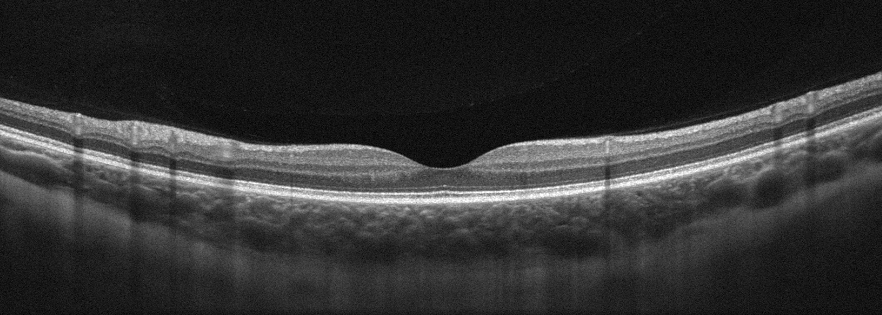
Left eye; OCT B-scan. The scan shows no evidence of AMD, DME, ERM, RAO, RVO, or VID.